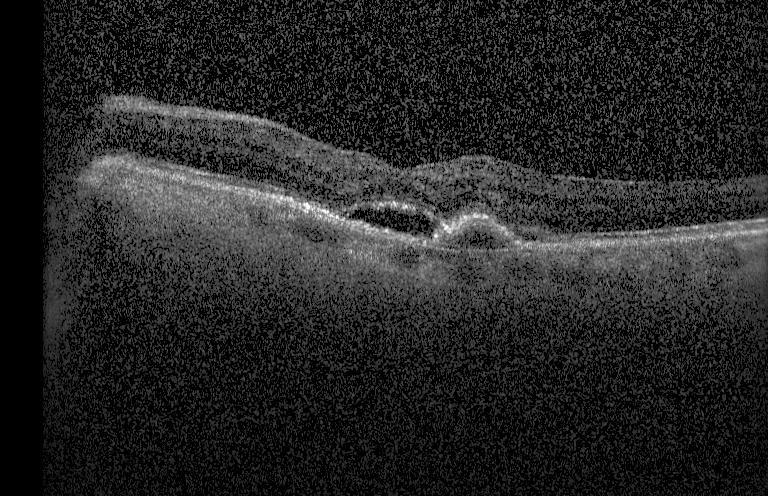

Impression: a choroidal neovascular membrane.